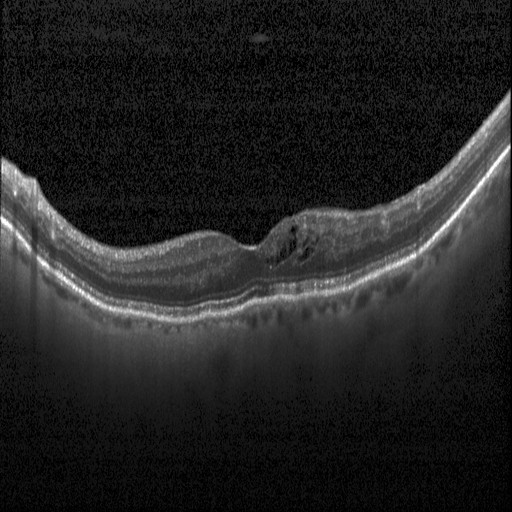
Retinal OCT cross-section — This B-scan demonstrates DME.